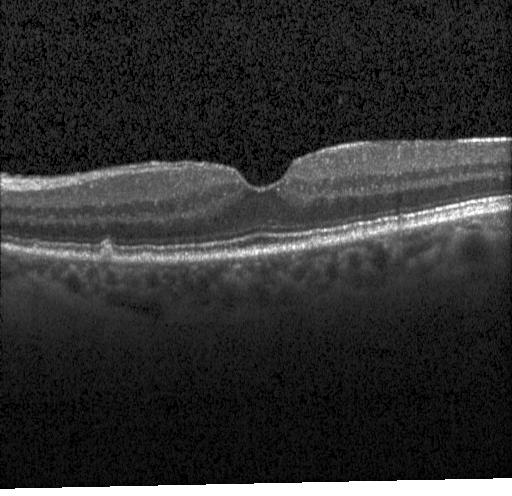

Diagnosis: sub-RPE drusenoid deposits.